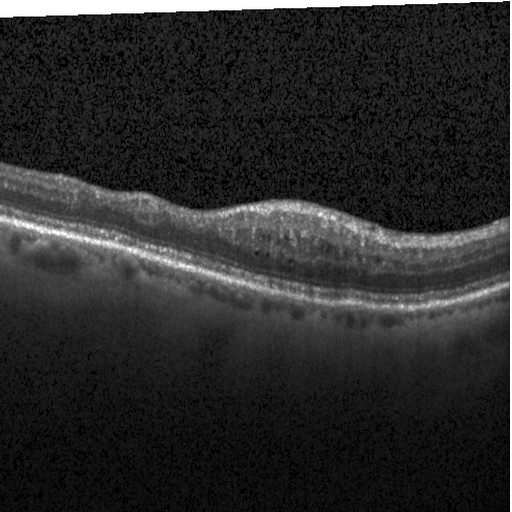
OCT line scan
Diagnosis: diabetic macular edema.